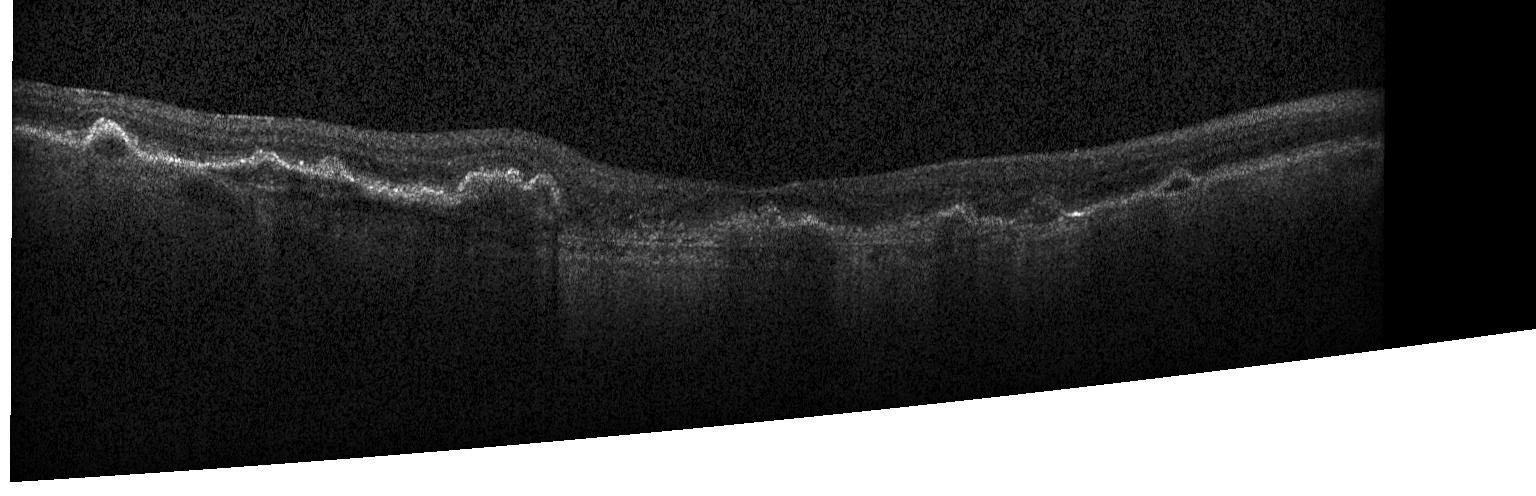 Dx: a choroidal neovascular membrane.